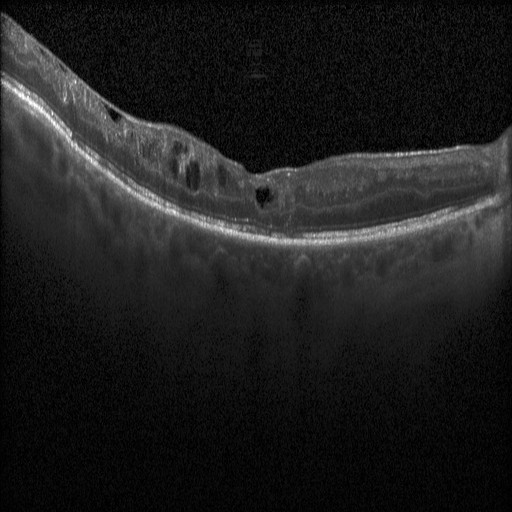 Horizontal scan through the fovea, retinal OCT cross-section — Impression: diabetic macular edema.